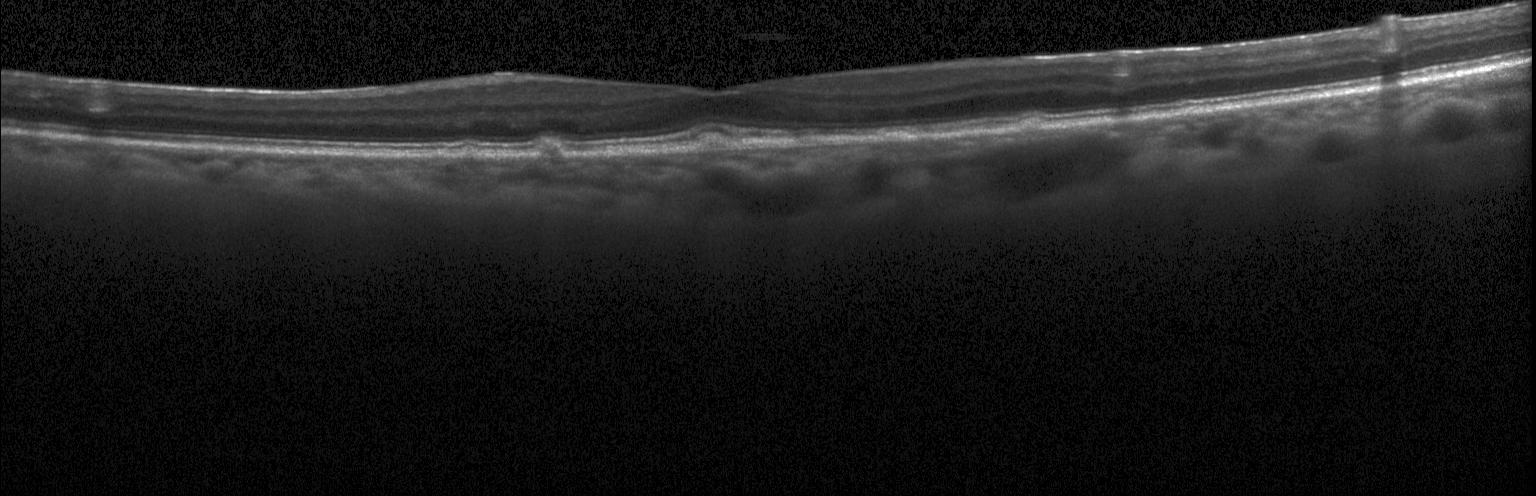

Through the macula. Heidelberg Spectralis OCT system. Optical coherence tomography B-scan. Spectral-domain OCT — This B-scan demonstrates multiple drusen.